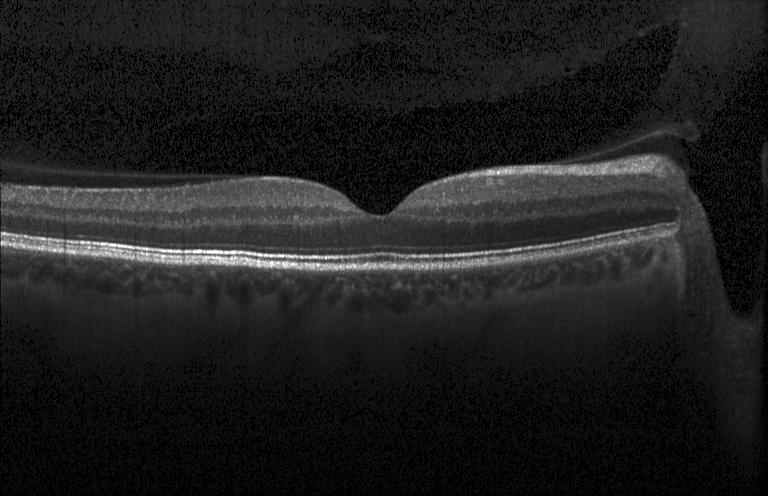

Impression: neither CNV, DME, nor drusen.